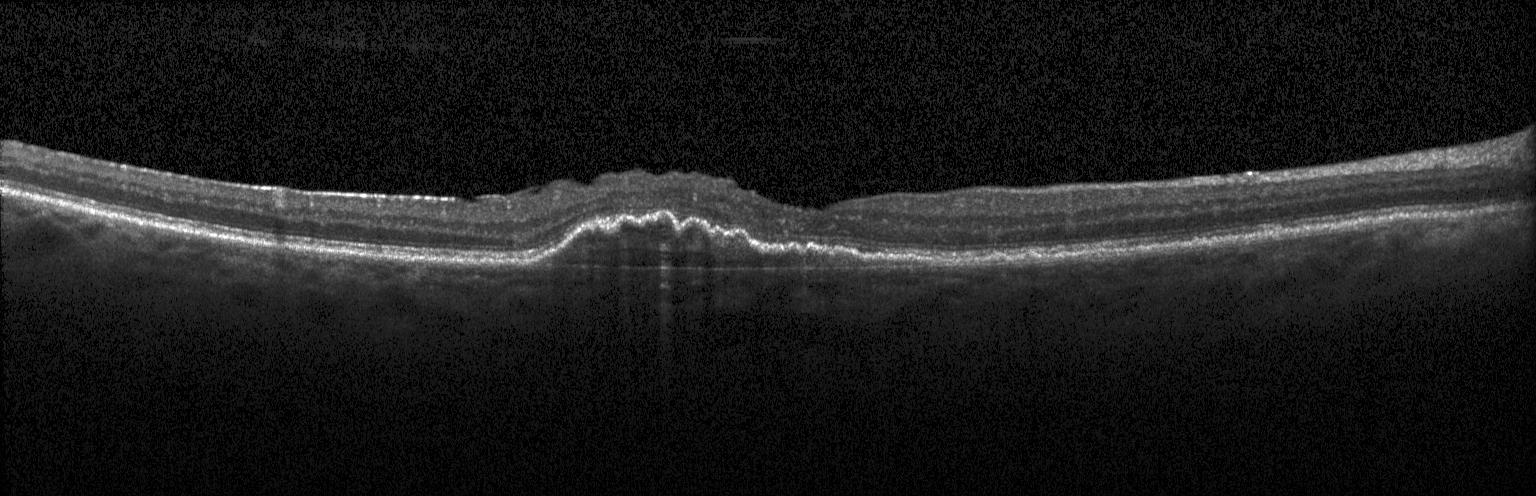

Through the macula. OCT B-scan. Acquired on a Heidelberg Spectralis. Finding: a choroidal neovascular membrane.